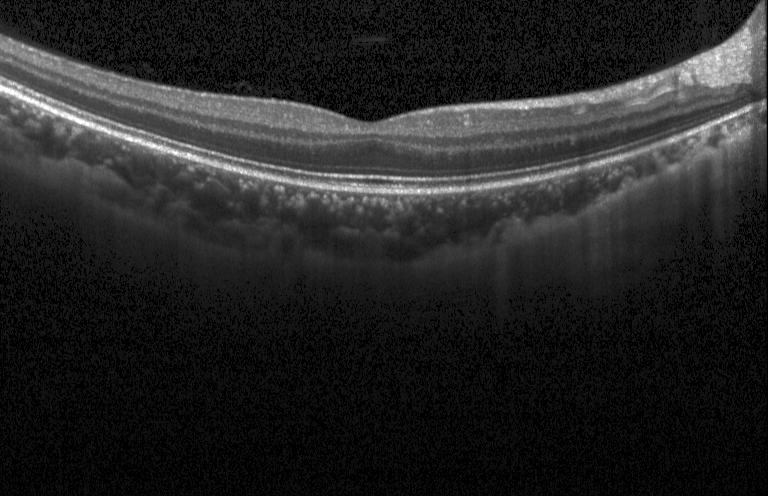
Diagnosis: no CNV, no DME, and no drusen.